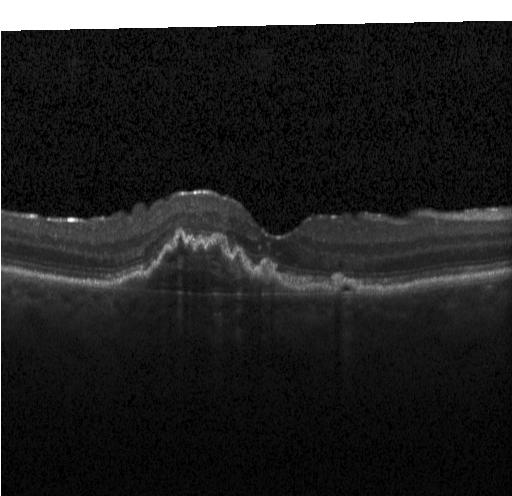
Through the macula. Acquired on a Heidelberg Spectralis. Optical coherence tomography scan
Macular OCT: CNV.